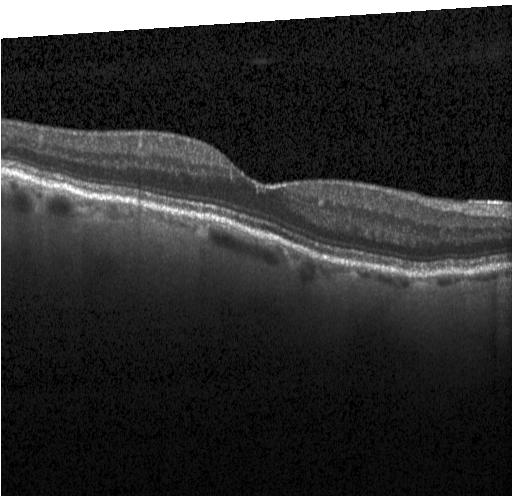

Optical coherence tomography B-scan · spectral-domain OCT
Assessment: no evidence of CNV, DME, or drusen.